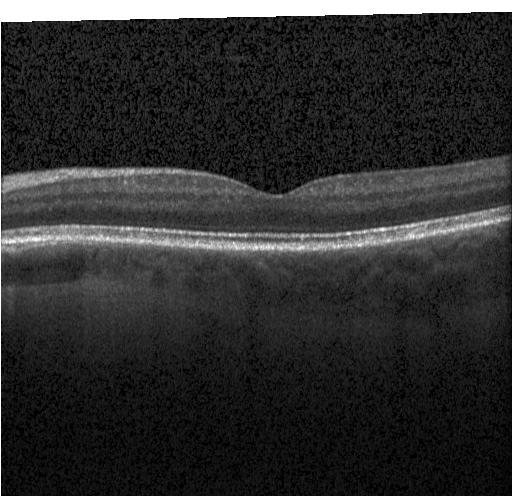
Spectral-domain OCT, retinal OCT B-scan. OCT finding: no choroidal neovascularization, diabetic macular edema, or drusen.